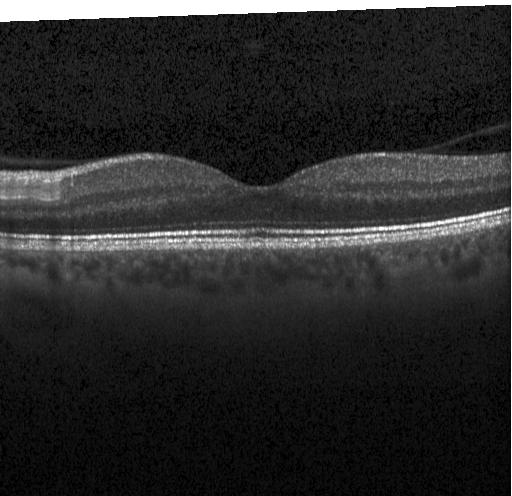
Horizontal scan through the fovea. Optical coherence tomography scan
No CNV, DME, or drusen.